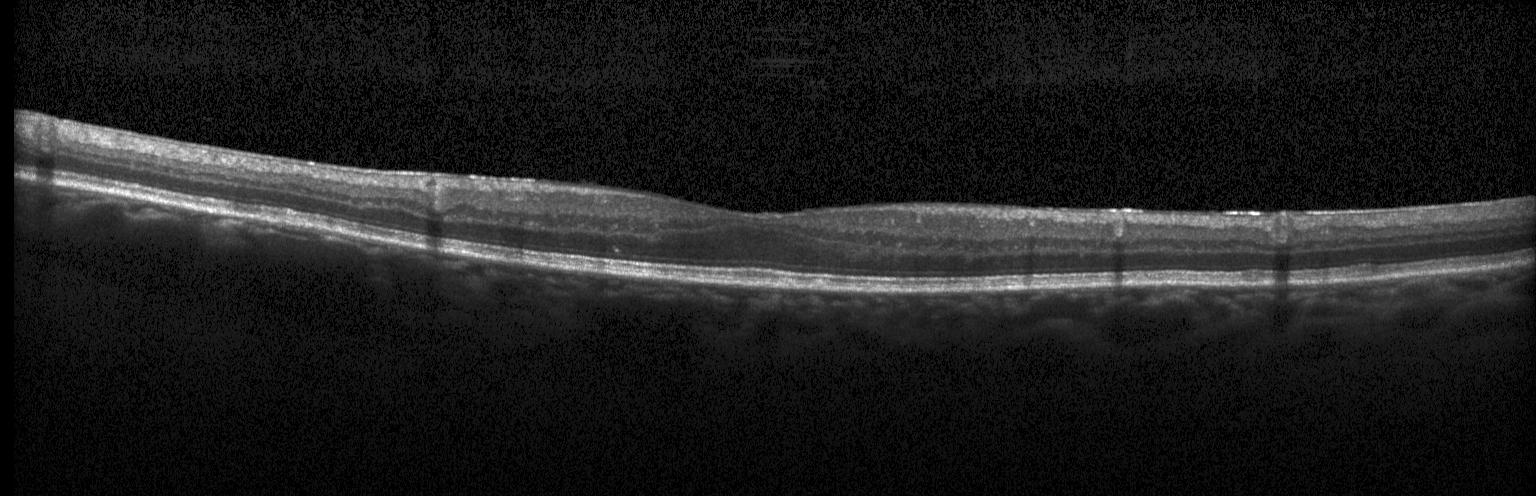

Impression: no evidence of choroidal neovascularization, diabetic macular edema, or drusen.